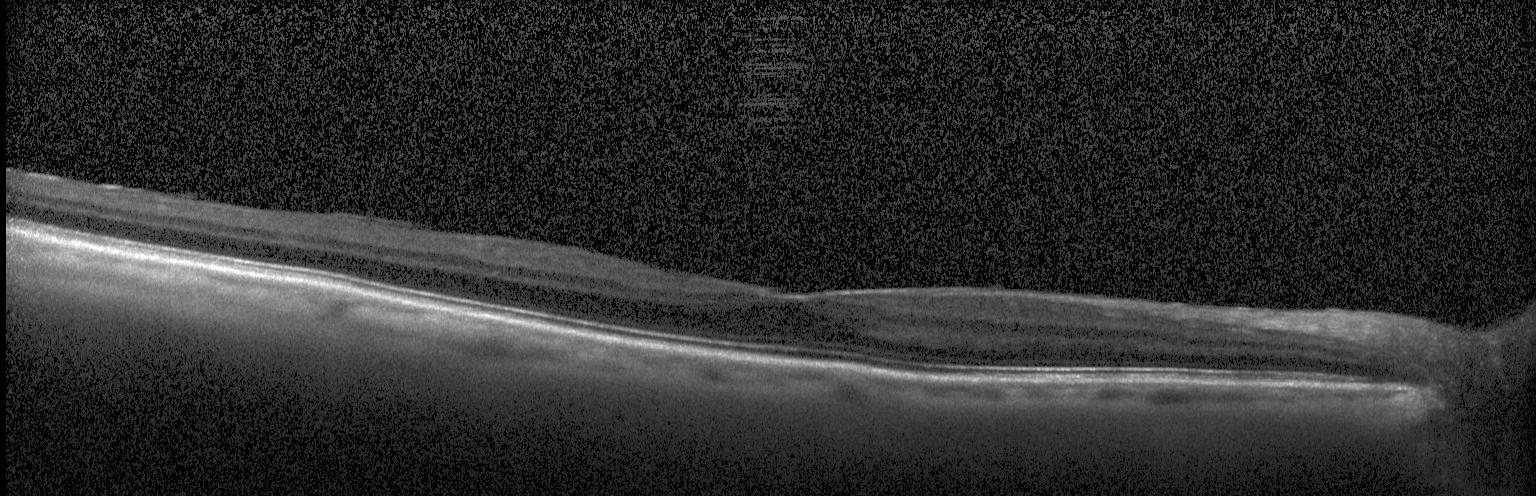

Centered on the fovea; acquired on a Heidelberg Spectralis; spectral-domain optical coherence tomography; optical coherence tomography scan.
OCT finding: neither choroidal neovascularization, diabetic macular edema, nor drusen.